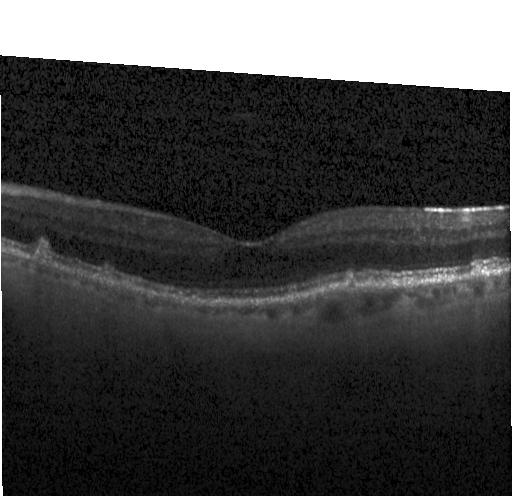
Spectral-domain OCT; optical coherence tomography B-scan. Assessment: drusen.